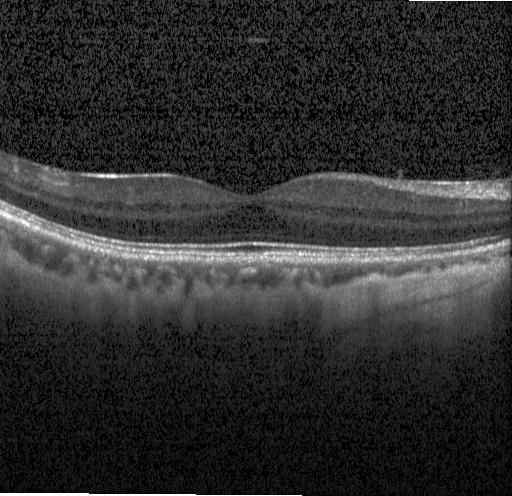
Retinal OCT B-scan; centered on the fovea; SD-OCT.
Finding: no choroidal neovascularization, no diabetic macular edema, and no drusen.